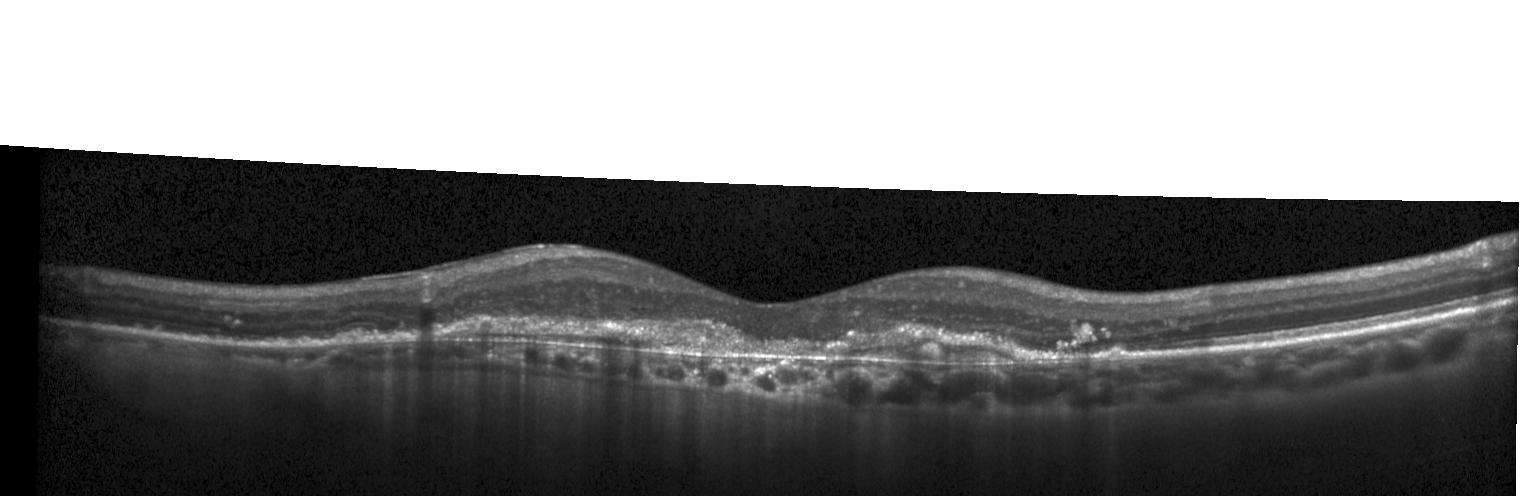 Through the macula, optical coherence tomography scan — OCT finding: CNV.